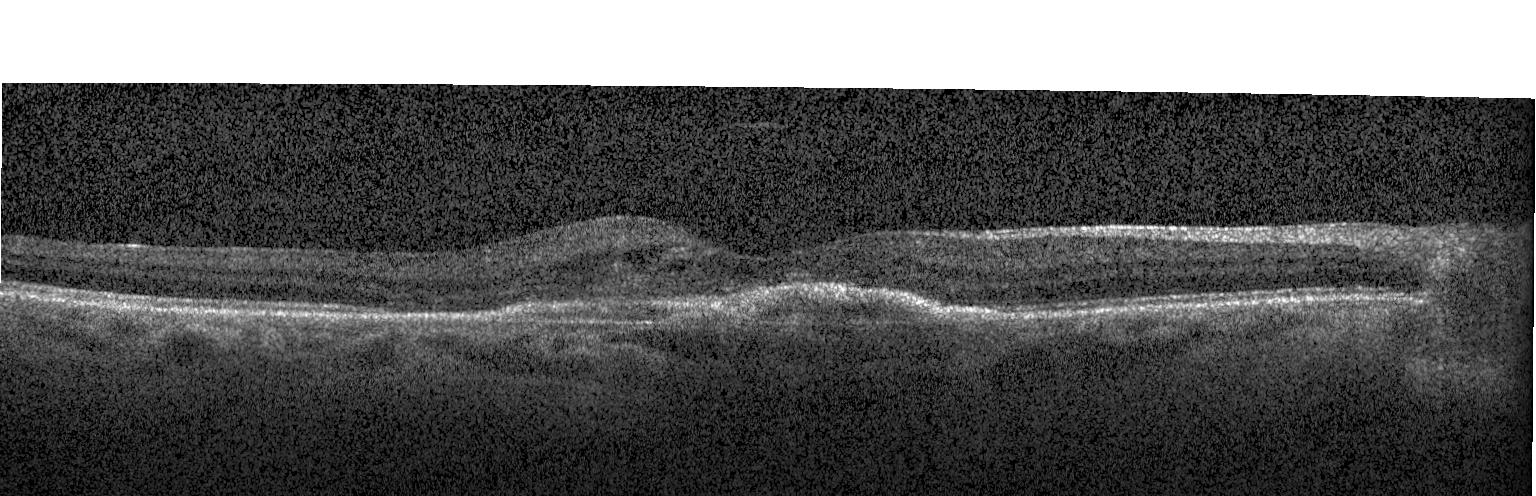

Macular OCT: choroidal neovascularization.